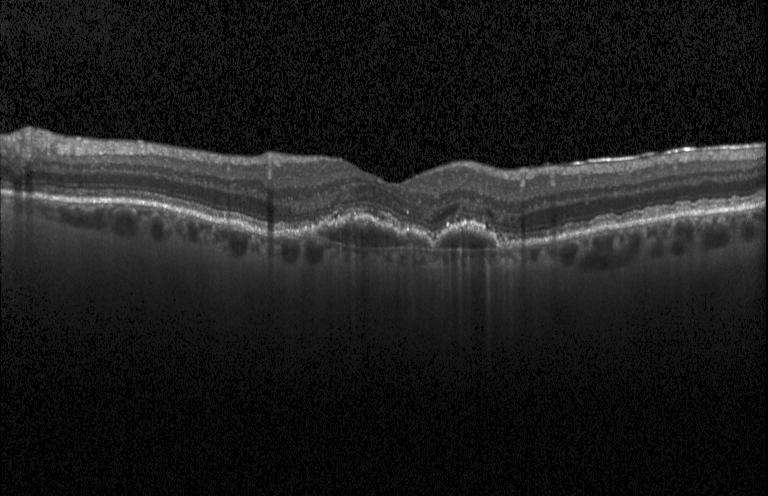 Macular OCT: a choroidal neovascular membrane.